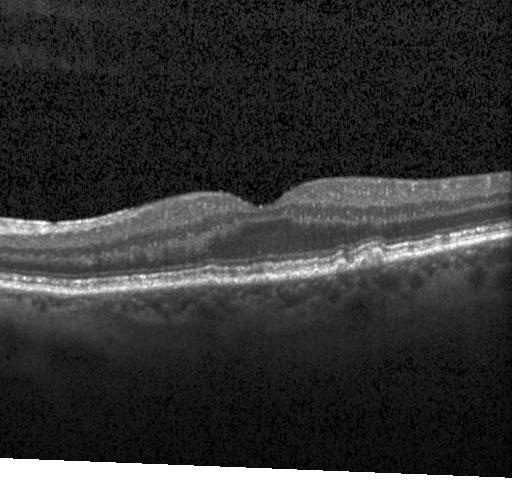

Macular OCT demonstrating multiple drusen.